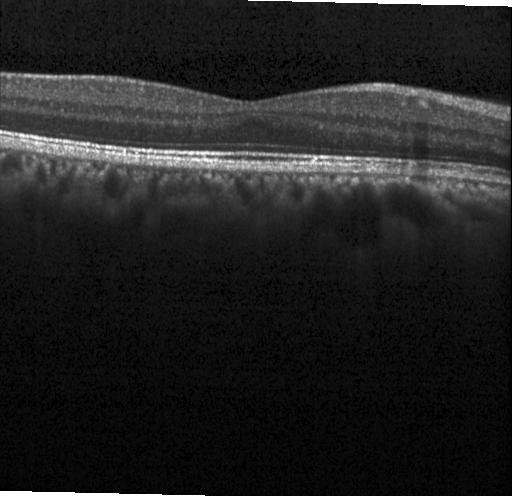 Centered on the fovea, spectral-domain OCT, retinal OCT B-scan, instrument: Heidelberg Spectralis. Neither choroidal neovascularization, diabetic macular edema, nor drusen.